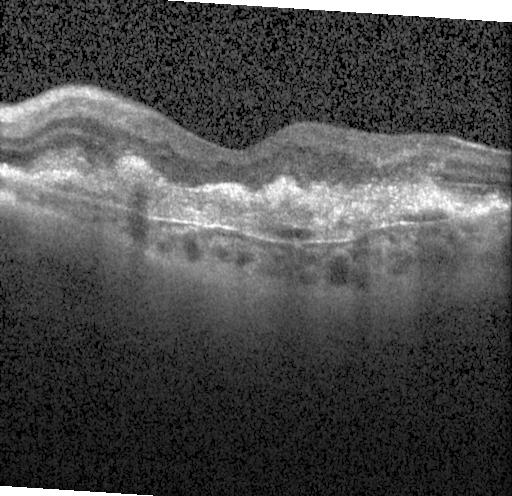
Optical coherence tomography scan — This B-scan demonstrates a choroidal neovascular membrane.